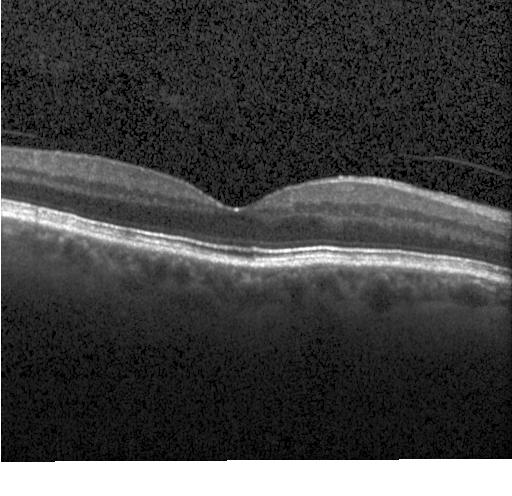 Dx: no CNV, DME, or drusen.